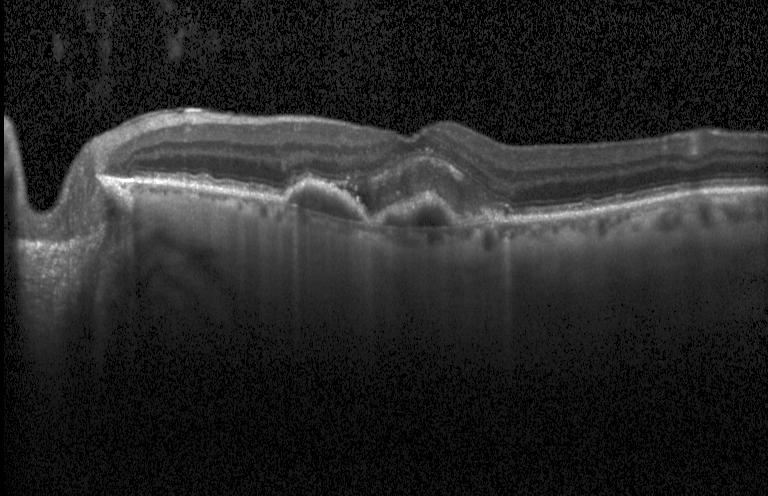 Acquired on a Heidelberg Spectralis. Optical coherence tomography B-scan
Finding: a choroidal neovascular membrane.